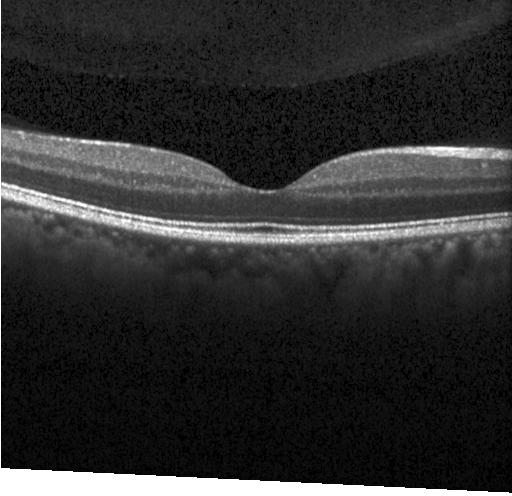

Spectral-domain OCT B-scan: no choroidal neovascularization, diabetic macular edema, or drusen.